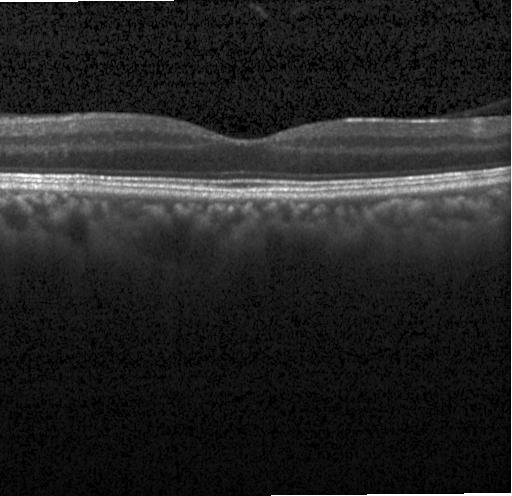

OCT line scan. Impression: neither CNV, DME, nor drusen.